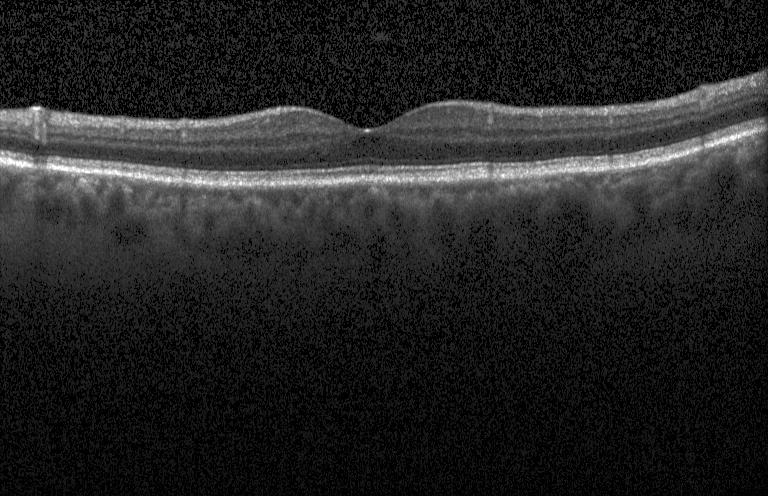 Finding: no choroidal neovascularization, no diabetic macular edema, and no drusen.